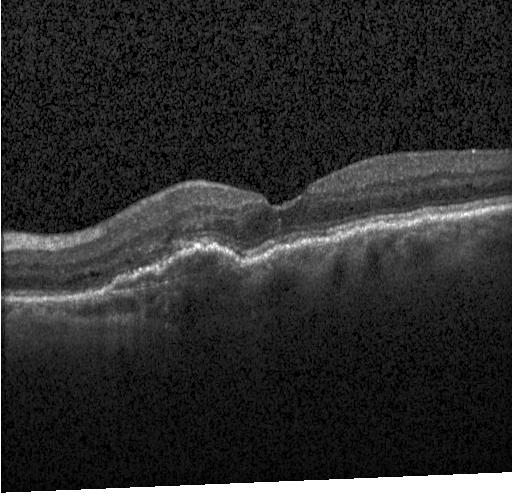 SD-OCT; retinal OCT cross-section; acquired on a Heidelberg Spectralis — Macular OCT: choroidal neovascularization (CNV).